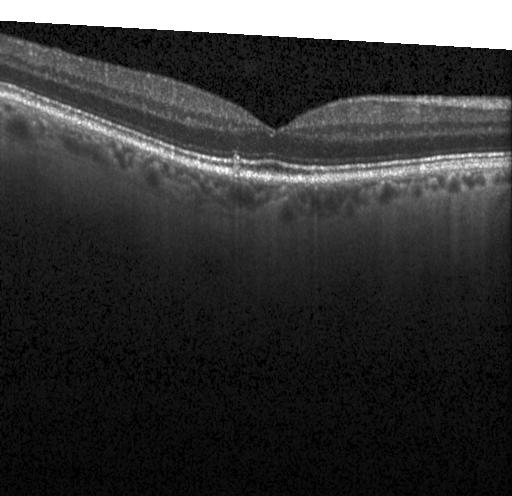
OCT B-scan · instrument: Heidelberg Spectralis. Assessment: no choroidal neovascularization, diabetic macular edema, or drusen.